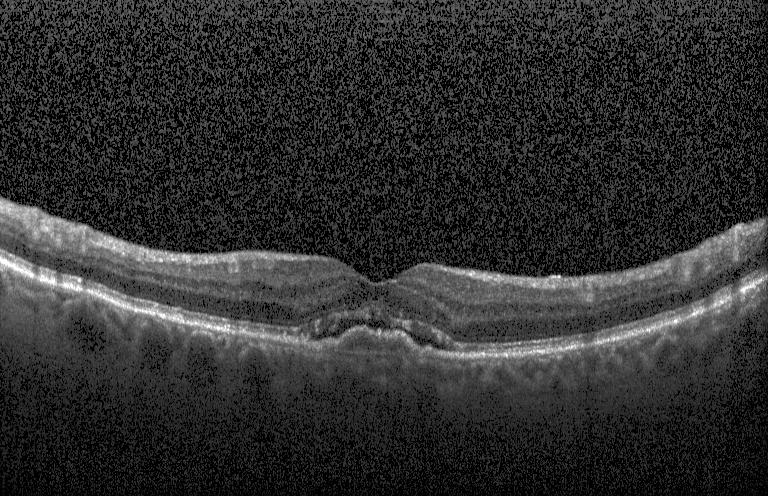 SD-OCT · OCT line scan
This B-scan demonstrates choroidal neovascularization.